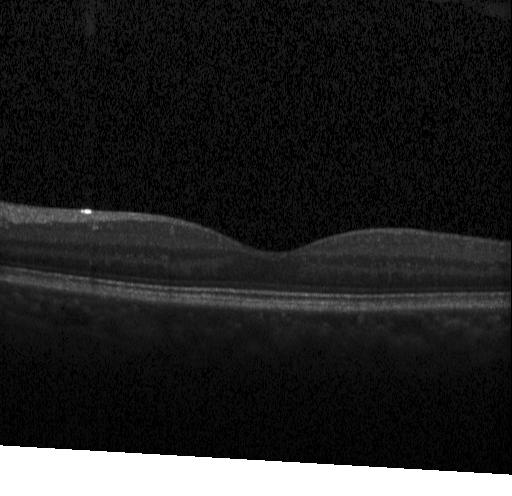
Retinal OCT B-scan — Neither choroidal neovascularization, diabetic macular edema, nor drusen.